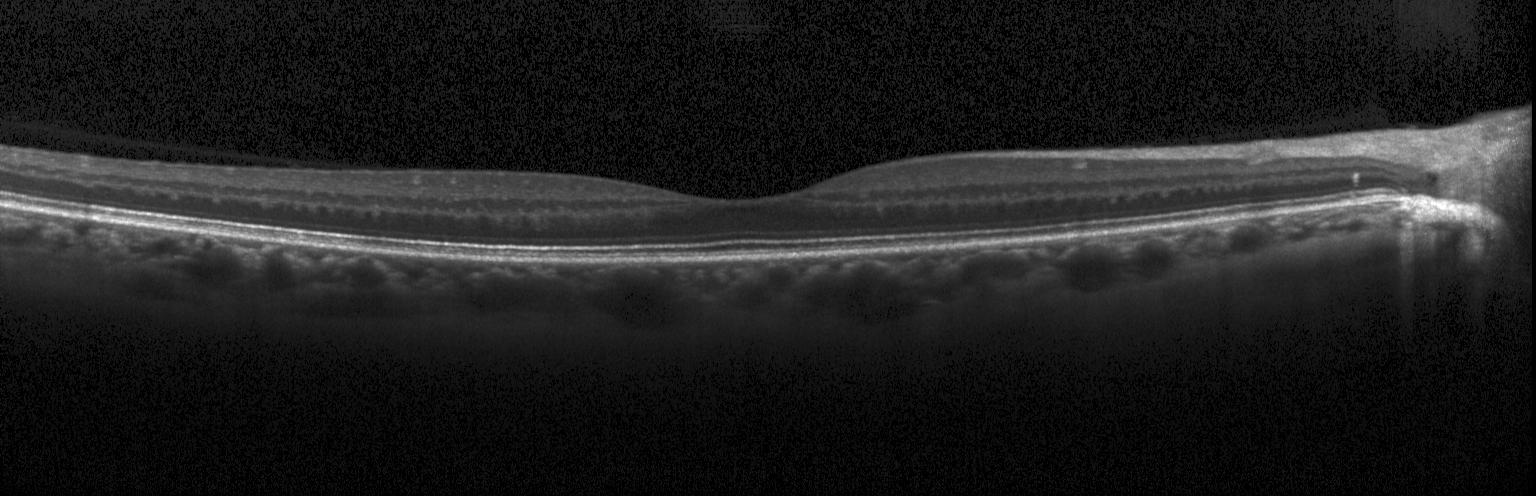
OCT line scan · centered on the fovea · SD-OCT. Finding: no evidence of CNV, DME, or drusen.